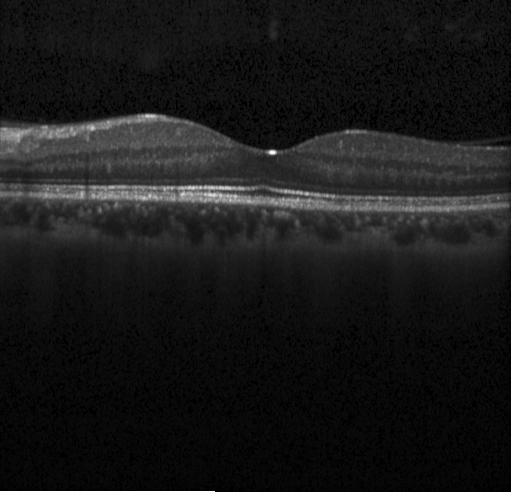
Diagnosis: no choroidal neovascularization, diabetic macular edema, or drusen.